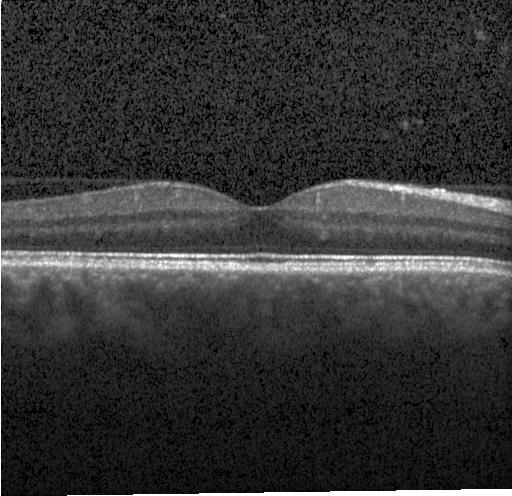
Retinal OCT cross-section
Dx: no CNV, DME, or drusen.